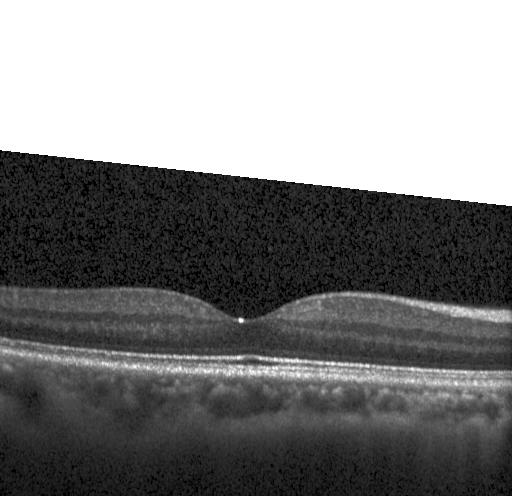

Heidelberg Spectralis OCT system · optical coherence tomography scan
The scan shows neither CNV, DME, nor drusen.